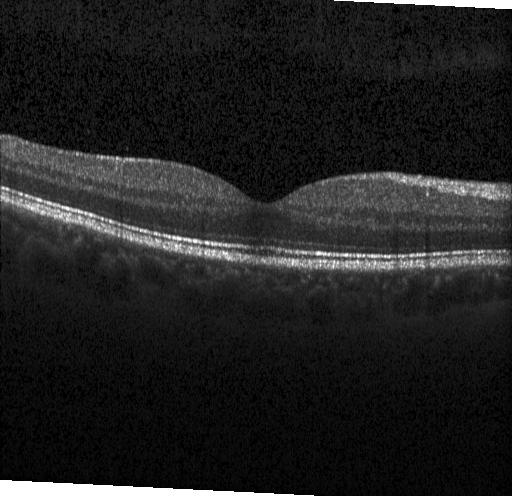
Optical coherence tomography B-scan, Heidelberg Spectralis, horizontal scan through the fovea, spectral-domain optical coherence tomography — Diagnosis: no evidence of choroidal neovascularization, diabetic macular edema, or drusen.